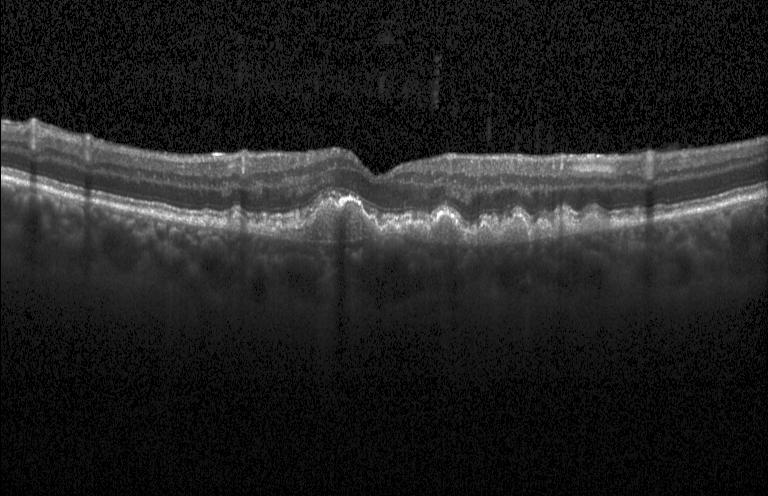 Heidelberg Spectralis · OCT B-scan
Finding: CNV.